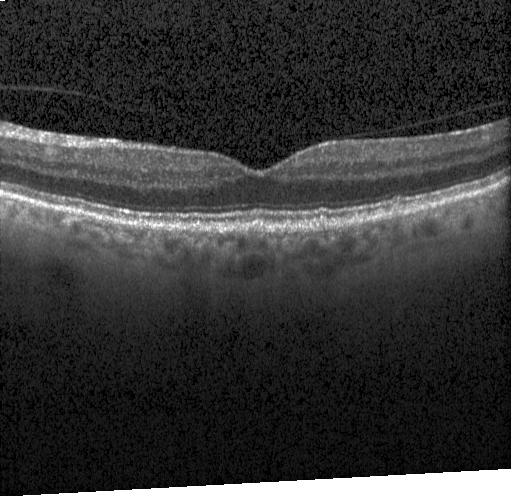
Centered on the fovea; retinal OCT B-scan — Finding: drusen.